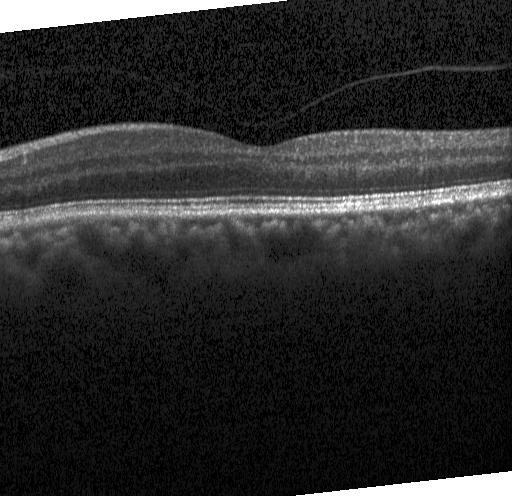 Fovea-centered; Heidelberg Spectralis; SD-OCT; OCT line scan
OCT finding: no evidence of CNV, DME, or drusen.